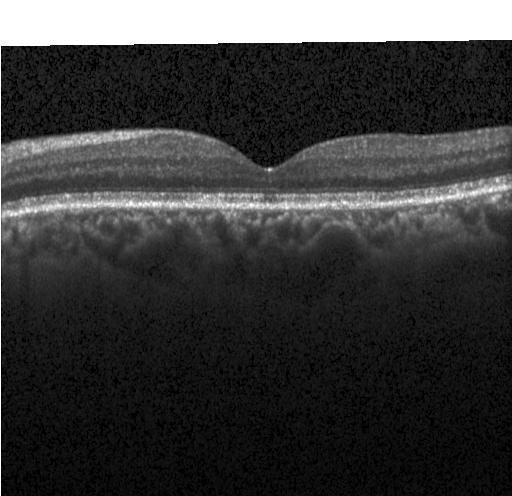

Retinal OCT B-scan
Dx: no choroidal neovascularization, diabetic macular edema, or drusen.